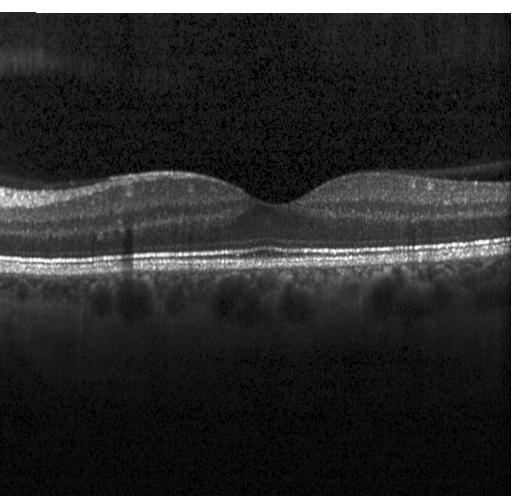
Spectral-domain optical coherence tomography; centered on the fovea; optical coherence tomography scan.
Diagnosis: no evidence of CNV, DME, or drusen.